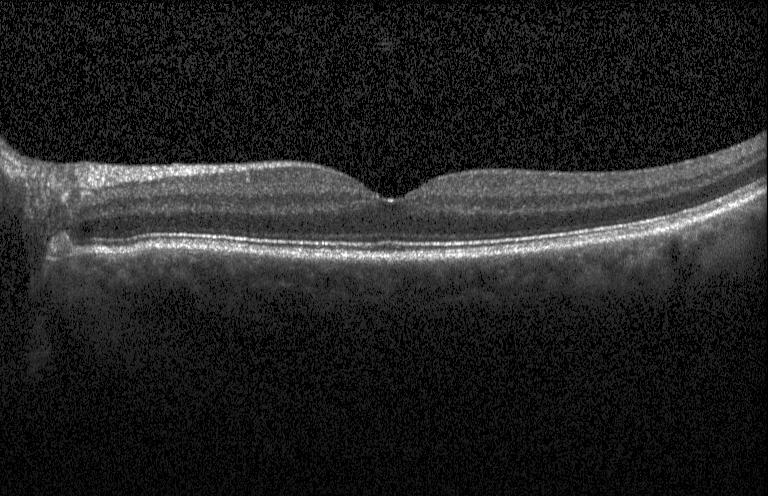 SD-OCT, retinal OCT cross-section, macular scan, Heidelberg Spectralis. The scan shows neither CNV, DME, nor drusen.